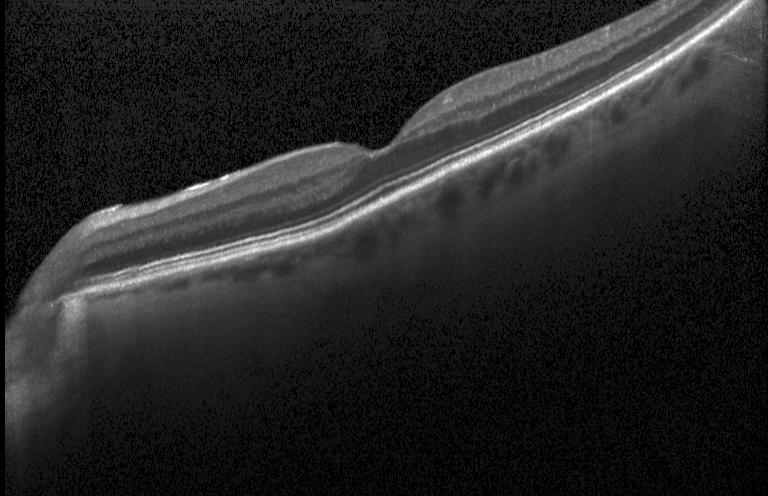

Optical coherence tomography B-scan.
Assessment: no evidence of choroidal neovascularization, diabetic macular edema, or drusen.